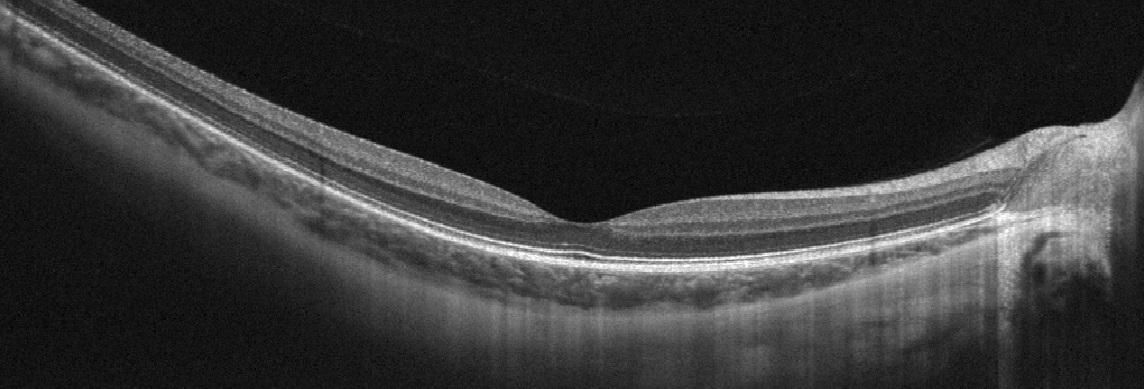 Macular OCT: absence of AMD, DME, ERM, RAO, RVO, and vitreomacular interface disease.